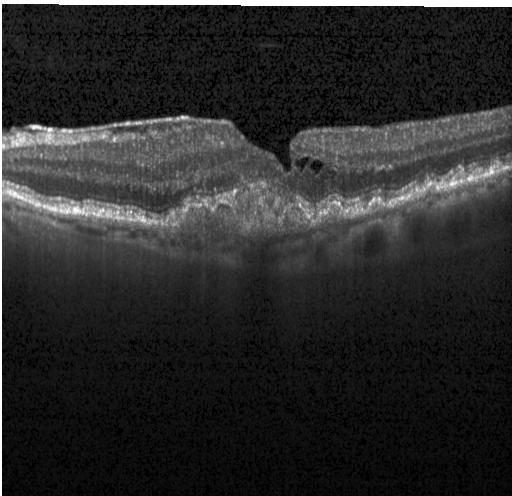 Retinal OCT cross-section. Spectral-domain OCT — Finding: choroidal neovascularization.